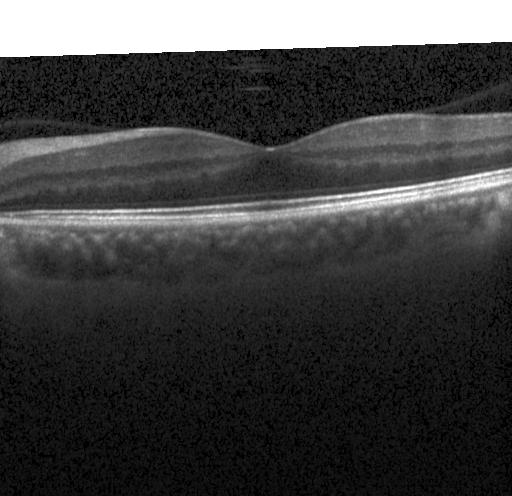 OCT B-scan · fovea-centered · Heidelberg Spectralis · spectral-domain OCT. No CNV, no DME, and no drusen.